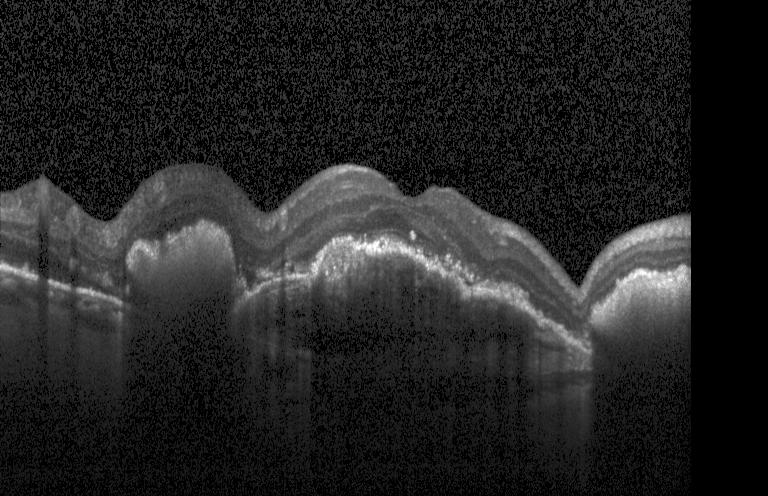 The scan shows a choroidal neovascular membrane.